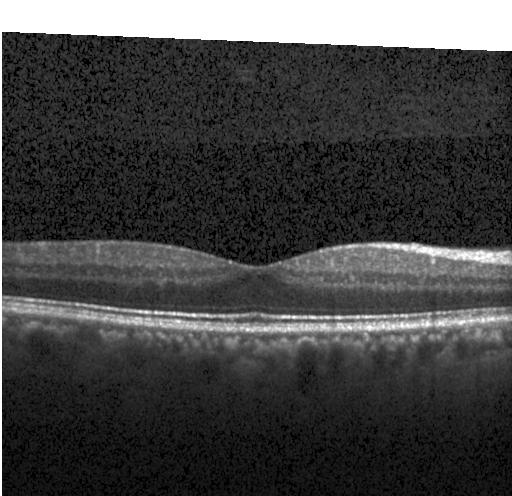 Heidelberg Spectralis · retinal OCT B-scan · spectral-domain optical coherence tomography — No choroidal neovascularization, diabetic macular edema, or drusen.